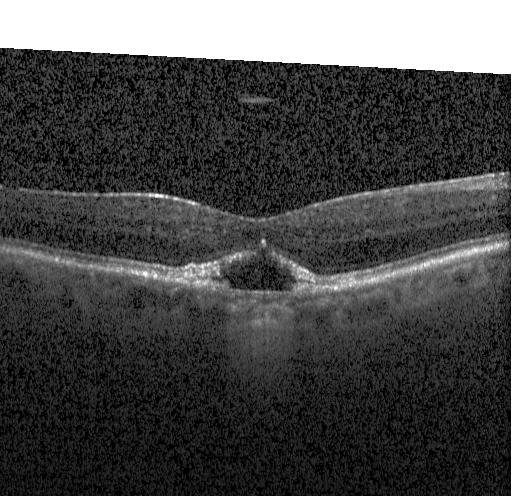
Optical coherence tomography B-scan · Heidelberg Spectralis OCT system · fovea-centered. Assessment: CNV.